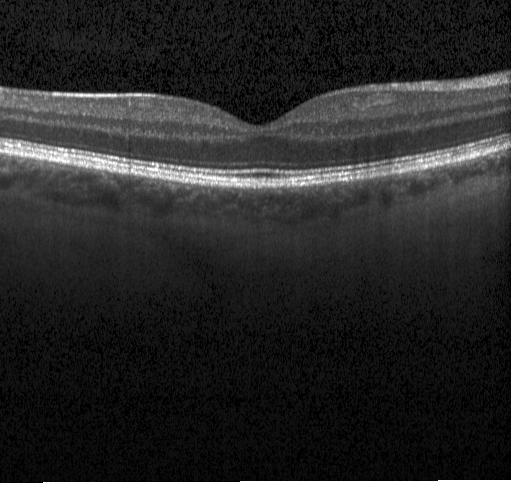 Finding: neither CNV, DME, nor drusen.